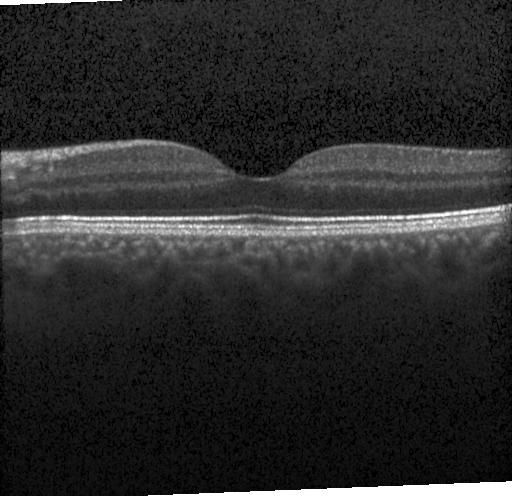
Heidelberg Spectralis OCT system · spectral-domain OCT · OCT B-scan. Dx: no CNV, DME, or drusen.